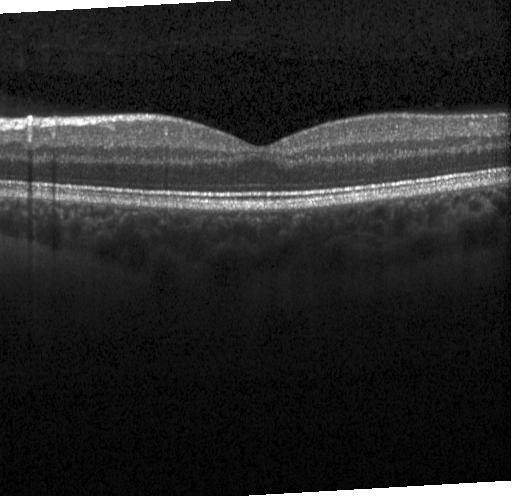

Heidelberg Spectralis. Through the macula. SD-OCT. OCT B-scan — Diagnosis: no evidence of choroidal neovascularization, diabetic macular edema, or drusen.